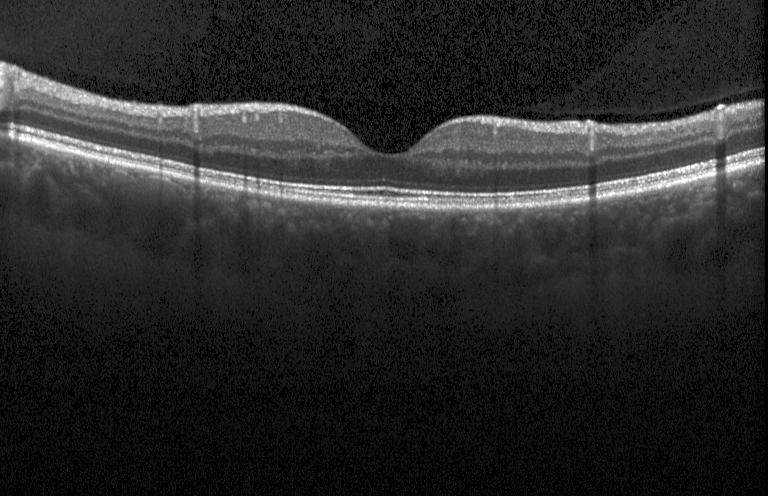 Finding: no choroidal neovascularization, no diabetic macular edema, and no drusen.